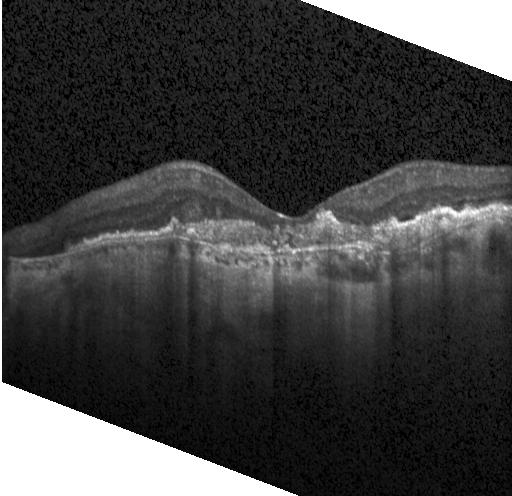

This B-scan demonstrates CNV.